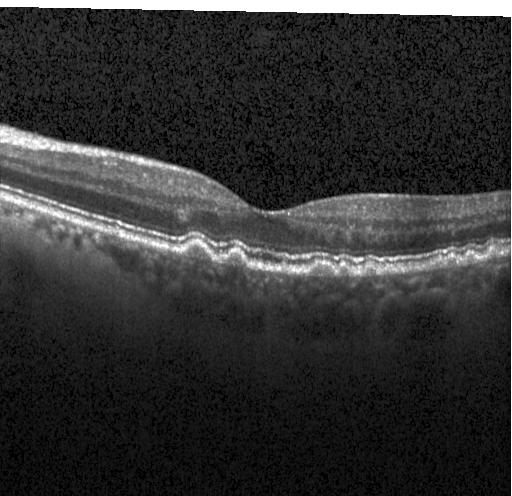

Fovea-centered; acquired on a Heidelberg Spectralis; SD-OCT; optical coherence tomography B-scan. Dx: drusen.